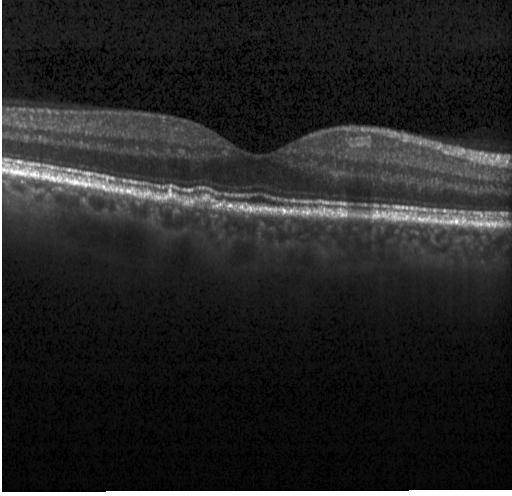
OCT scan showing sub-RPE drusenoid deposits.